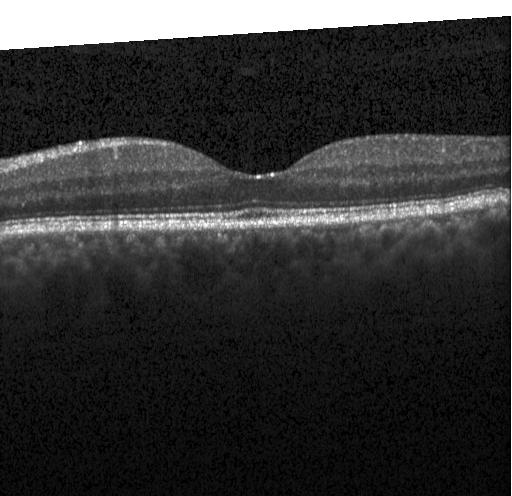

OCT B-scan showing no evidence of CNV, DME, or drusen.